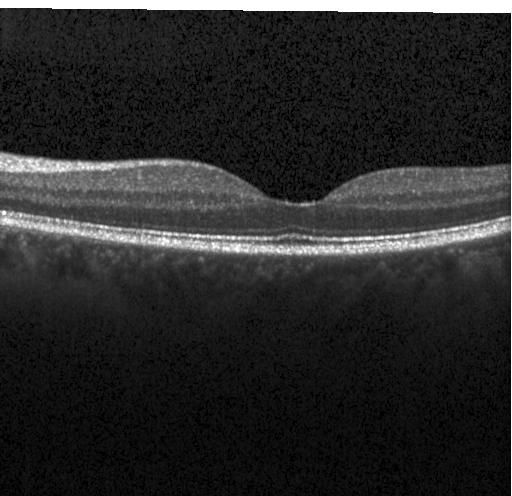 Retinal OCT cross-section · SD-OCT · through the macula
This B-scan demonstrates neither choroidal neovascularization, diabetic macular edema, nor drusen.